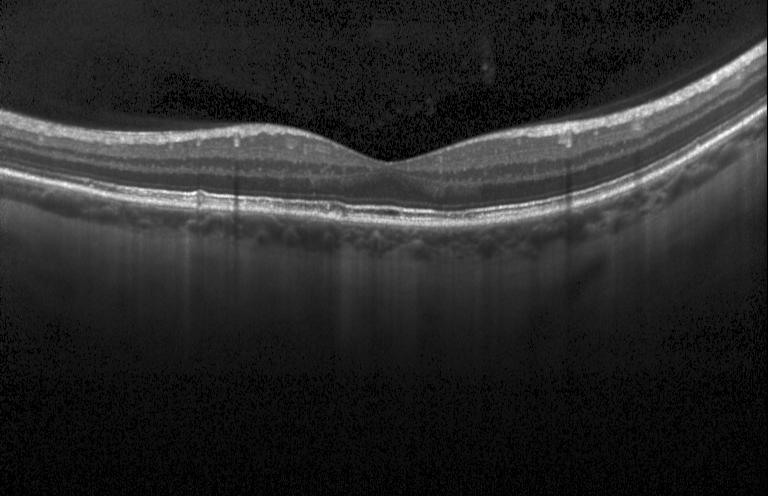 Macular OCT: neither choroidal neovascularization, diabetic macular edema, nor drusen.